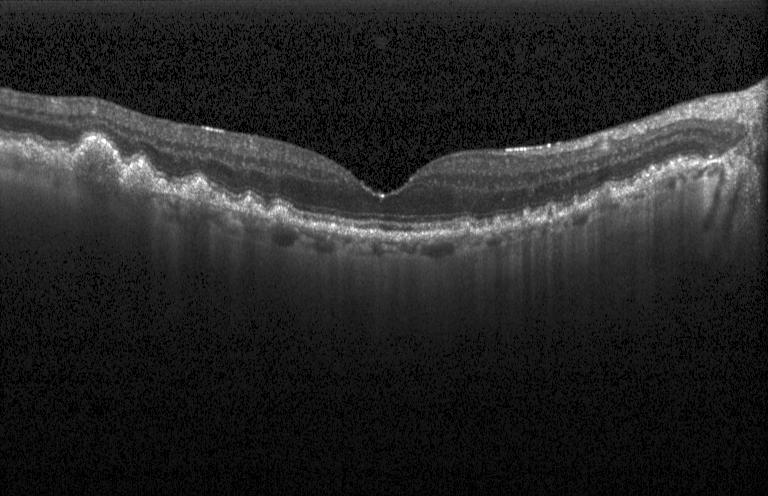
OCT line scan; Heidelberg Spectralis OCT system; SD-OCT — Impression: multiple drusen.